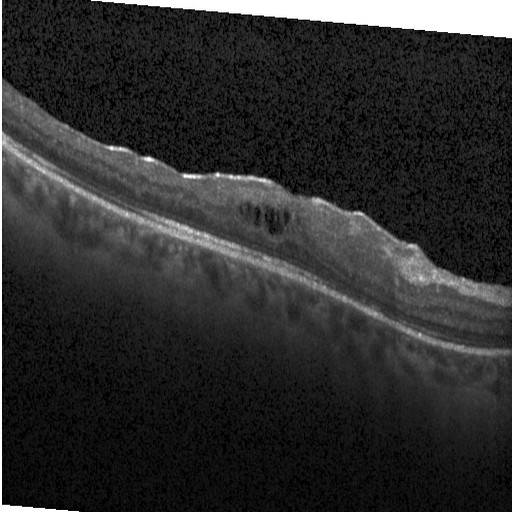 Instrument: Heidelberg Spectralis. Optical coherence tomography scan. Horizontal scan through the fovea.
Dx: DME.